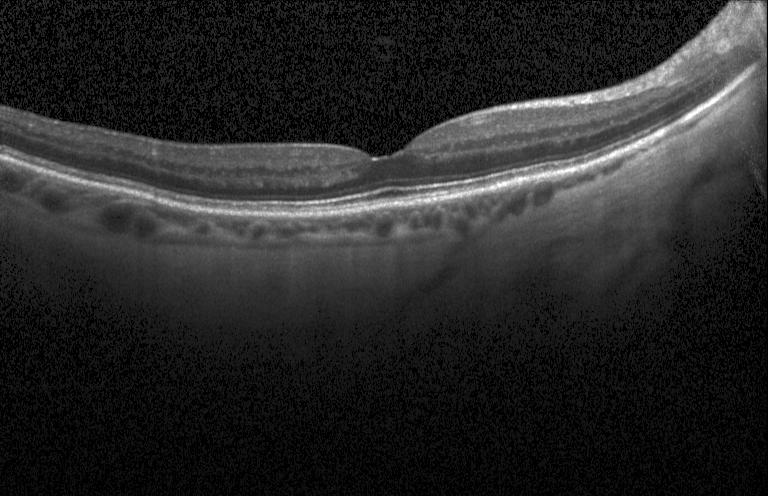

Neither choroidal neovascularization, diabetic macular edema, nor drusen.